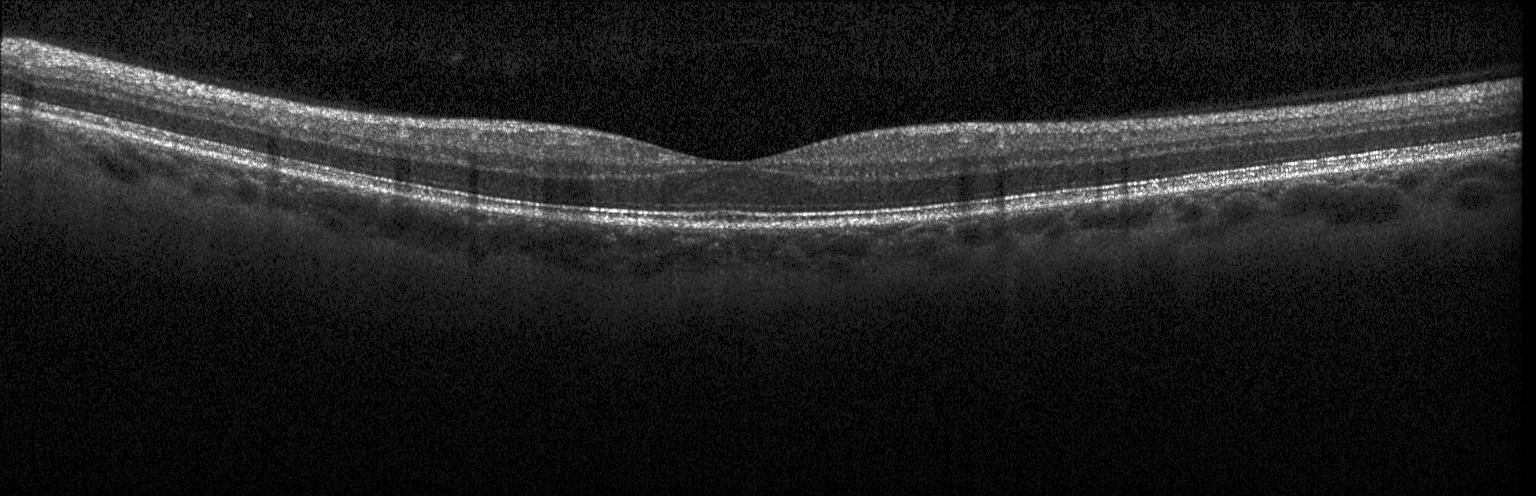
Spectral-domain OCT. Horizontal scan through the fovea. OCT B-scan. OCT finding: no evidence of CNV, DME, or drusen.